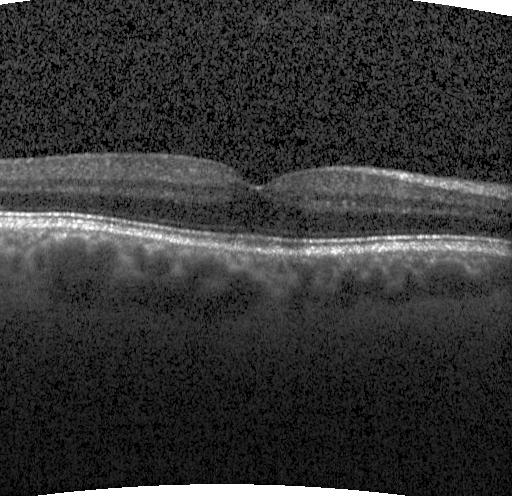

Instrument: Heidelberg Spectralis, OCT B-scan, through the macula.
The scan shows no evidence of choroidal neovascularization, diabetic macular edema, or drusen.